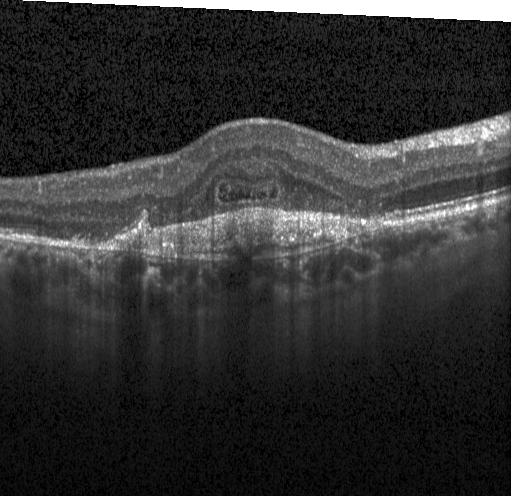

Impression: a choroidal neovascular membrane.